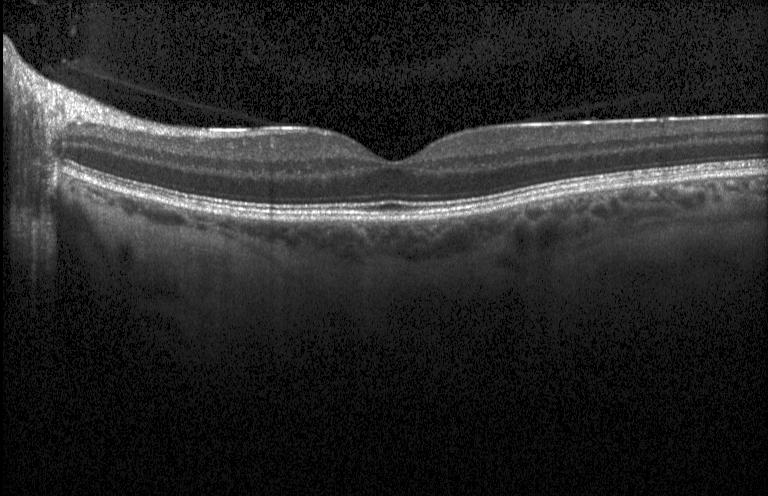

Impression: no CNV, DME, or drusen.